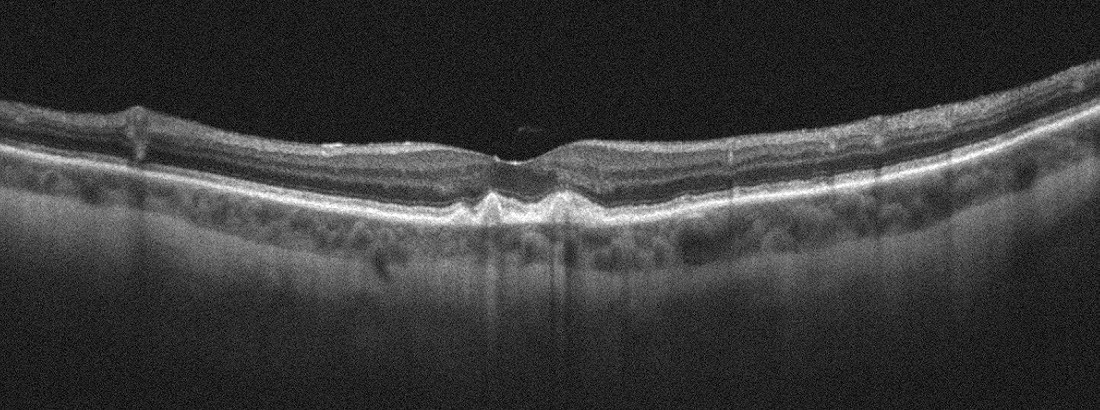
Retinal OCT B-scan. Macular OCT: age-related macular degeneration.